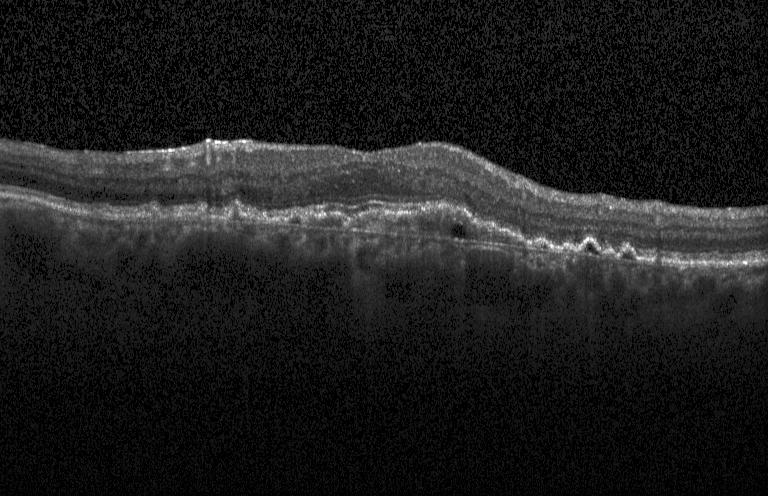
Optical coherence tomography scan. Impression: a choroidal neovascular membrane.